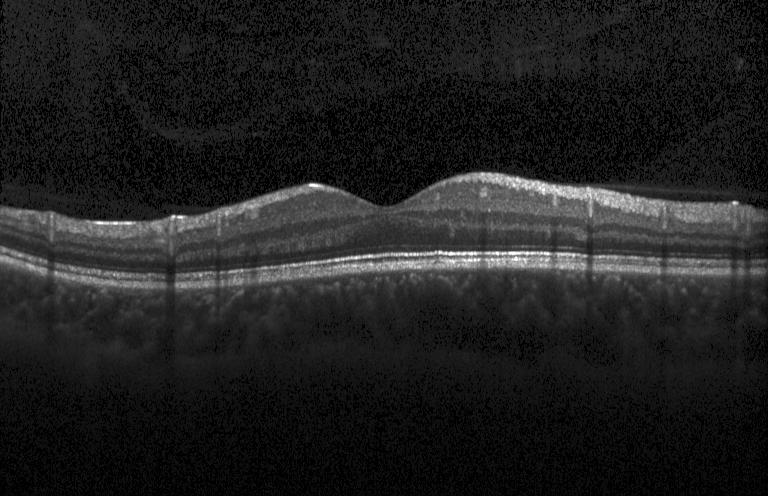
Impression: no choroidal neovascularization, no diabetic macular edema, and no drusen.